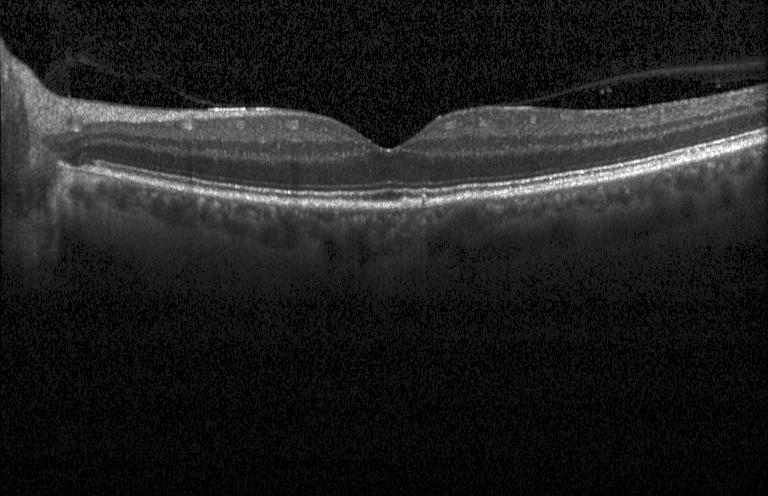
OCT B-scan, Heidelberg Spectralis OCT system, SD-OCT, horizontal scan through the fovea
Finding: neither choroidal neovascularization, diabetic macular edema, nor drusen.